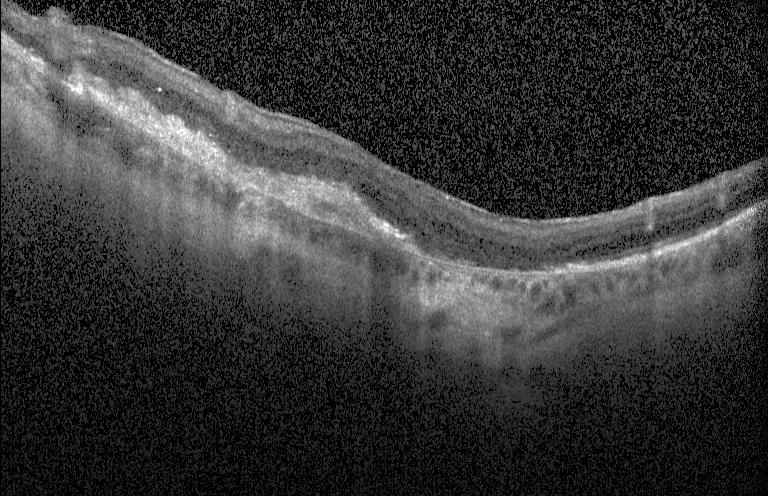 The scan shows choroidal neovascularization.